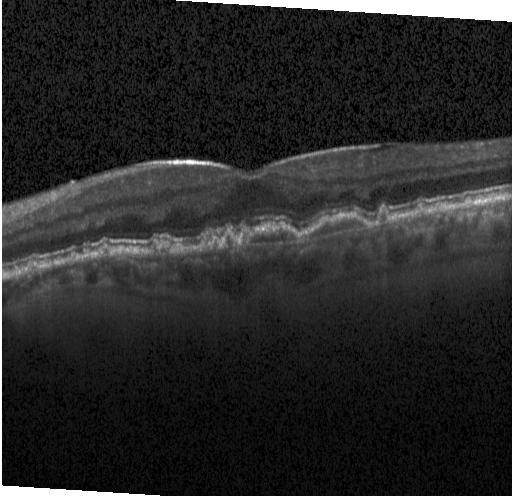
Finding: sub-RPE drusenoid deposits.